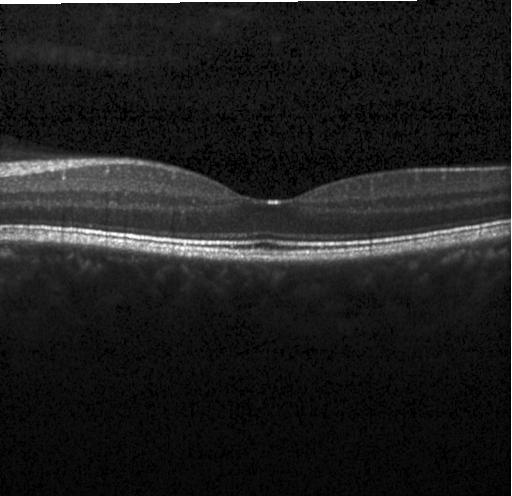

OCT B-scan showing neither choroidal neovascularization, diabetic macular edema, nor drusen.